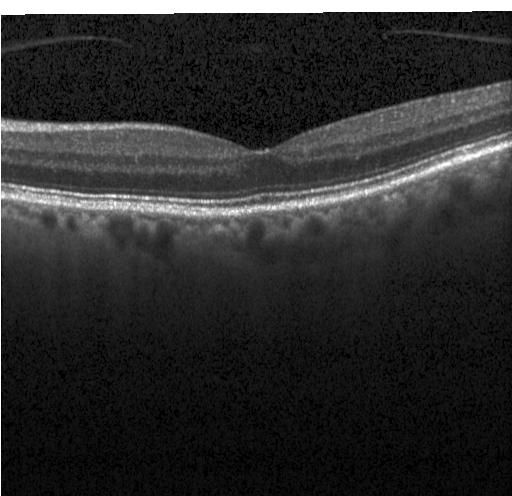 This B-scan demonstrates no choroidal neovascularization, diabetic macular edema, or drusen.